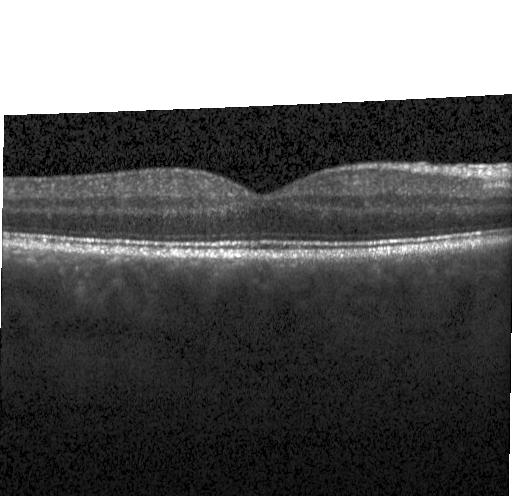

OCT line scan; spectral-domain OCT; acquired on a Heidelberg Spectralis — Finding: no evidence of choroidal neovascularization, diabetic macular edema, or drusen.